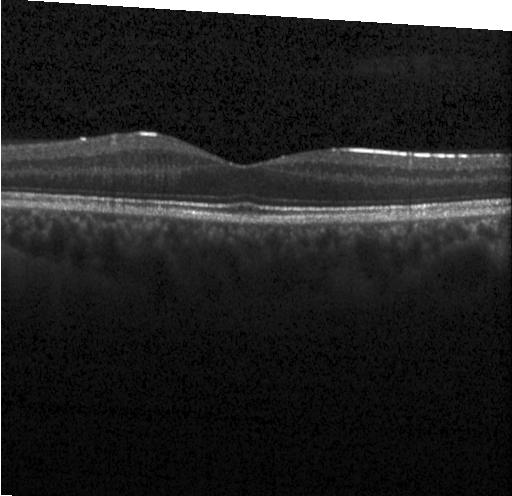
OCT B-scan showing neither choroidal neovascularization, diabetic macular edema, nor drusen.